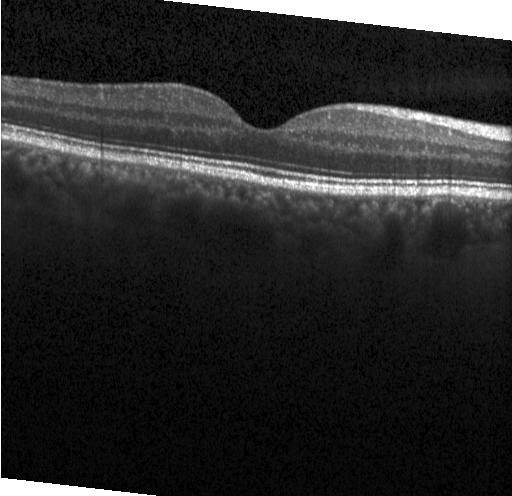
Impression: no evidence of choroidal neovascularization, diabetic macular edema, or drusen.